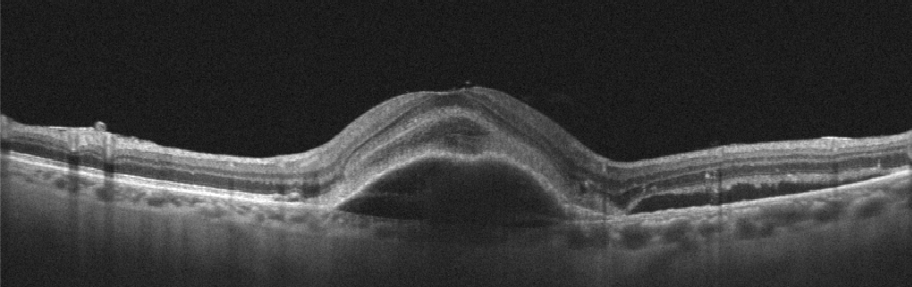 OCT B-scan.
Diagnosis: AMD.